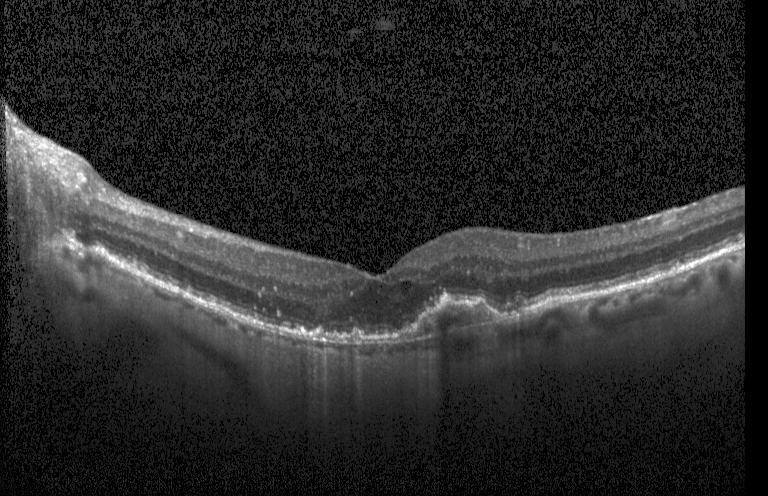

OCT line scan.
Impression: a choroidal neovascular membrane.